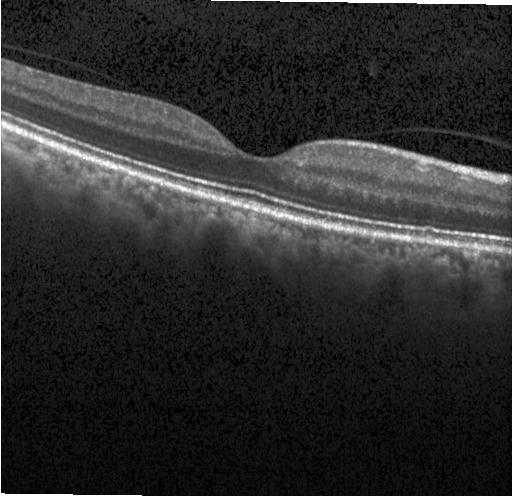
Macular OCT demonstrating no evidence of CNV, DME, or drusen.